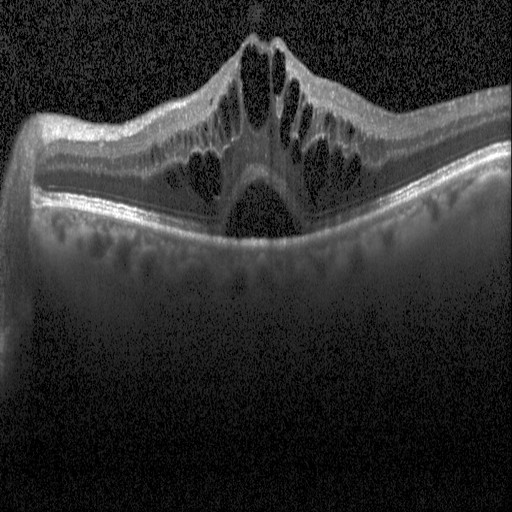

Diabetic macular edema.